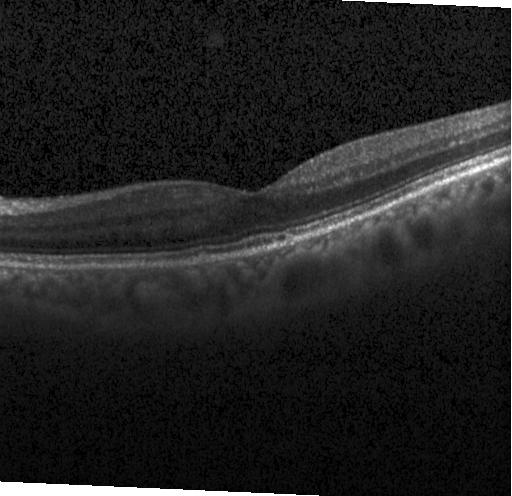
Multiple drusen.